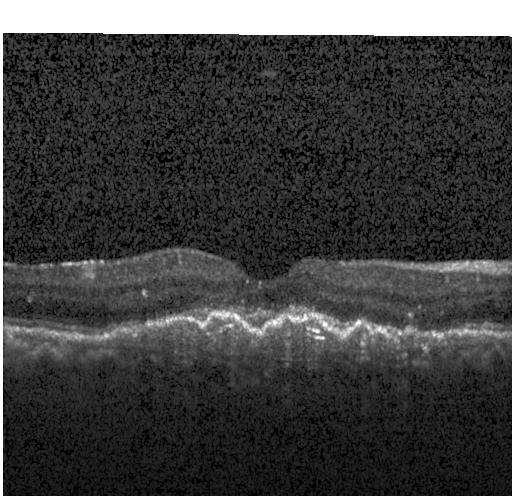
Dx: a choroidal neovascular membrane.